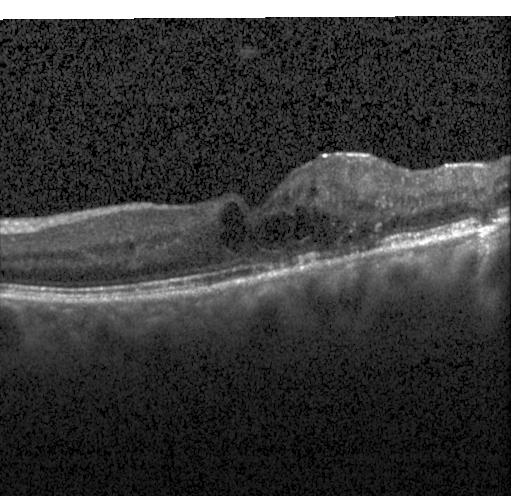
Assessment: DME.